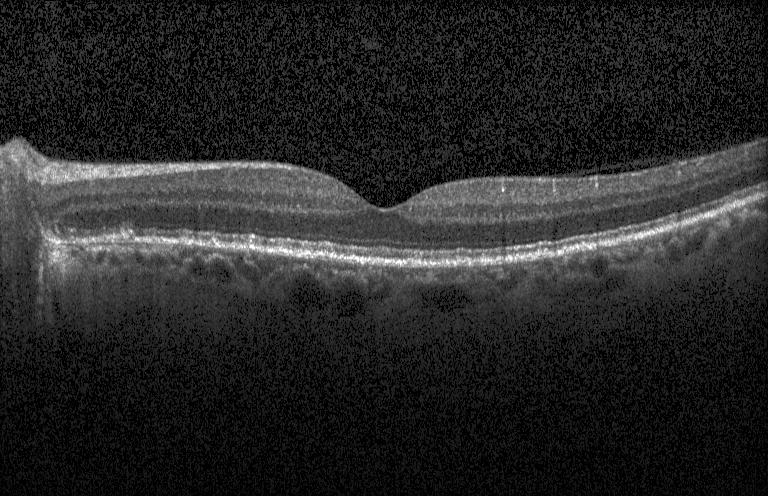 Optical coherence tomography B-scan — Diagnosis: no choroidal neovascularization, diabetic macular edema, or drusen.